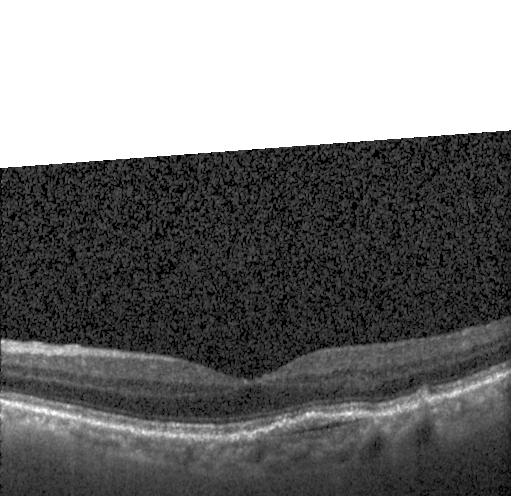 Optical coherence tomography B-scan — Impression: CNV.